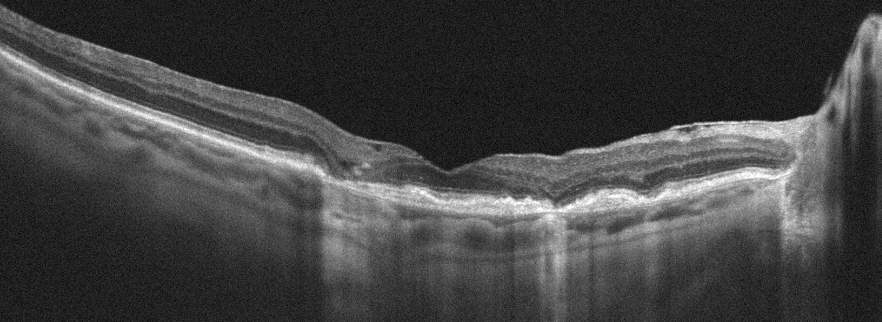 Acquired on an Optovue Avanti RTVue XR, OD, retinal OCT cross-section, through the macula
Dx: age-related macular degeneration.